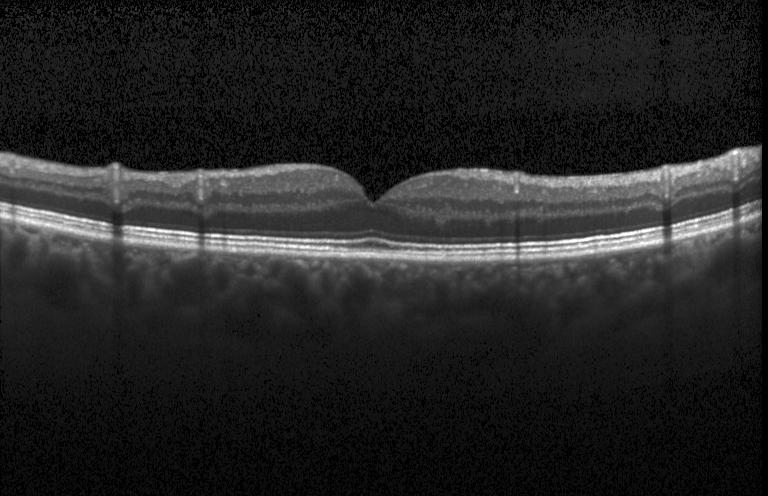 Retinal OCT cross-section showing no evidence of choroidal neovascularization, diabetic macular edema, or drusen.